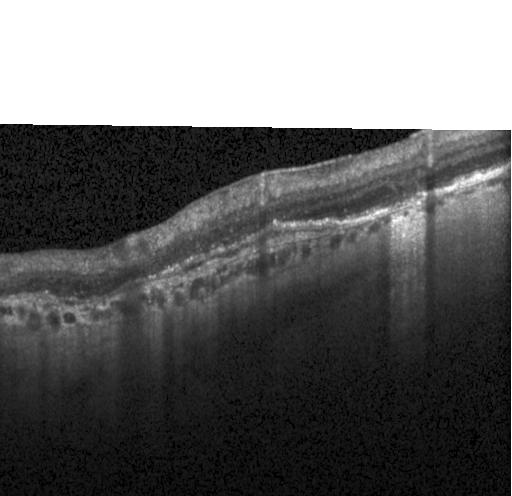

Macular OCT: choroidal neovascularization.